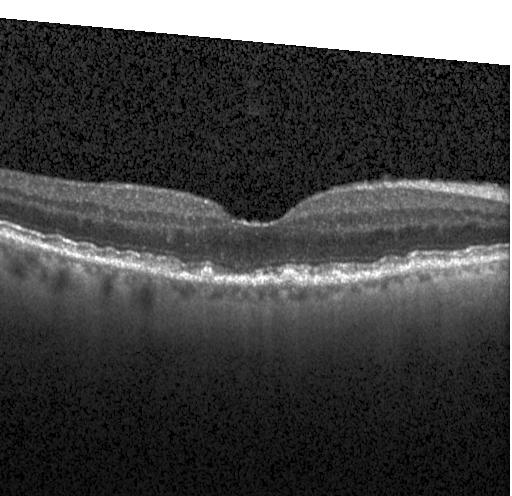
Retinal OCT cross-section — Impression: sub-RPE drusenoid deposits.